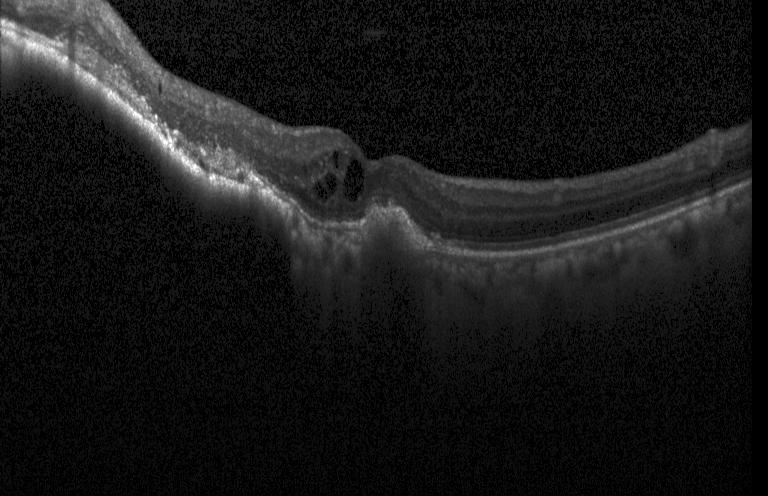 OCT line scan; spectral-domain optical coherence tomography; Heidelberg Spectralis OCT system; horizontal scan through the fovea
Diagnosis: a choroidal neovascular membrane.